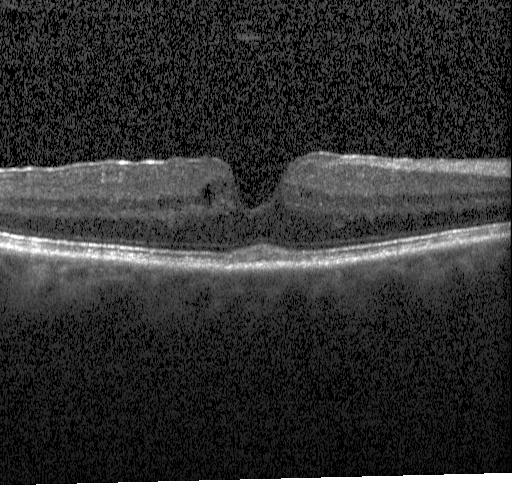

Macular scan. Heidelberg Spectralis OCT system. OCT B-scan
Impression: DME.